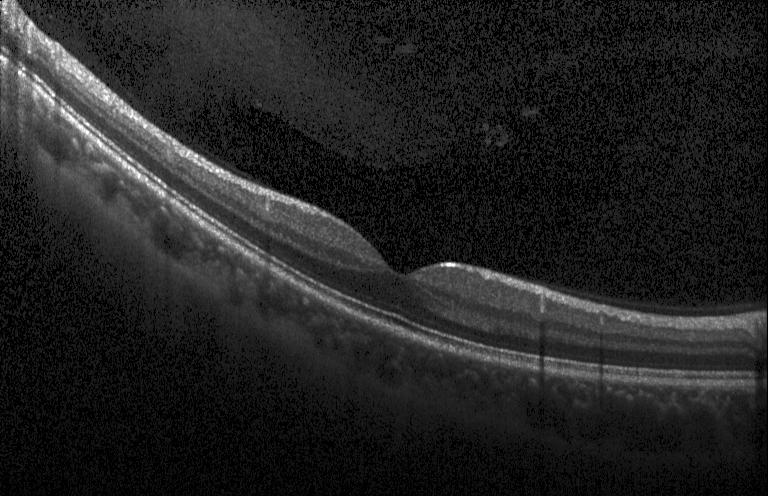 Diagnosis: neither choroidal neovascularization, diabetic macular edema, nor drusen.